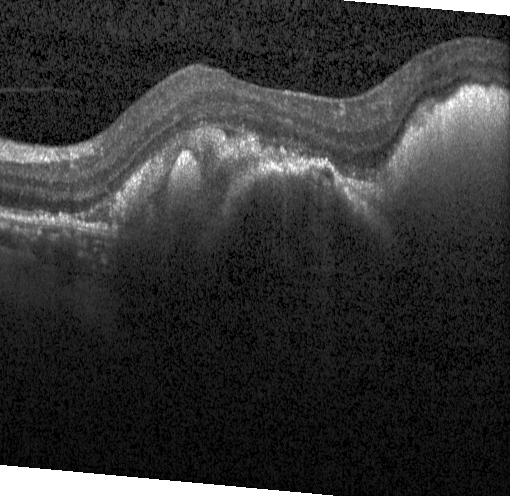

Dx: a choroidal neovascular membrane.